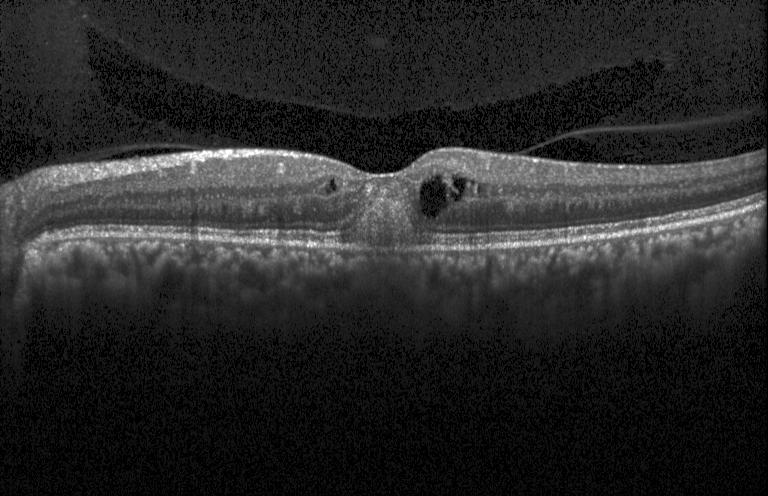
The scan shows a choroidal neovascular membrane.